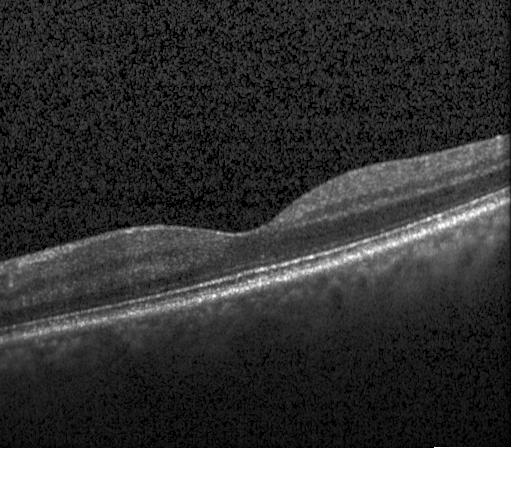

Impression: no evidence of CNV, DME, or drusen.